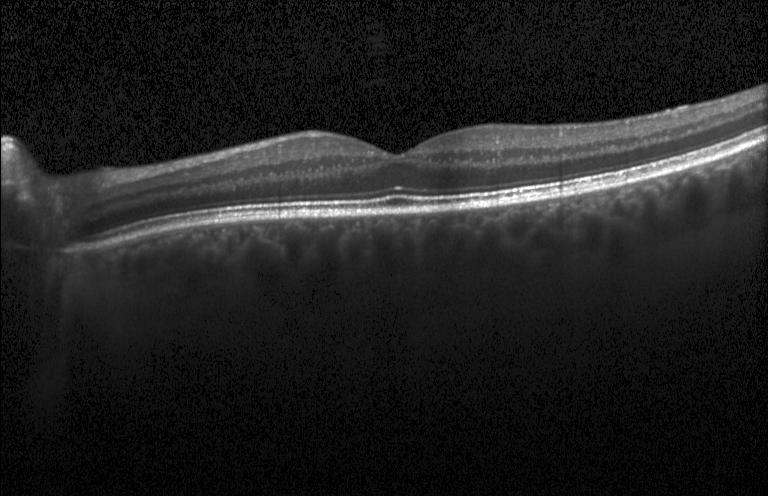 Acquired on a Heidelberg Spectralis, fovea-centered, OCT B-scan — Finding: no choroidal neovascularization, diabetic macular edema, or drusen.